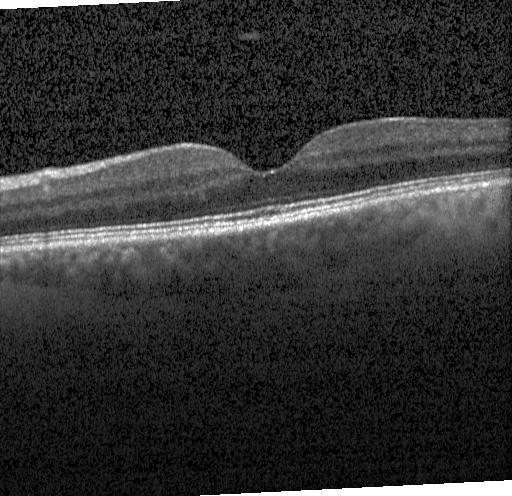 Optical coherence tomography B-scan. Macular scan. Heidelberg Spectralis OCT system.
Diagnosis: no choroidal neovascularization, diabetic macular edema, or drusen.